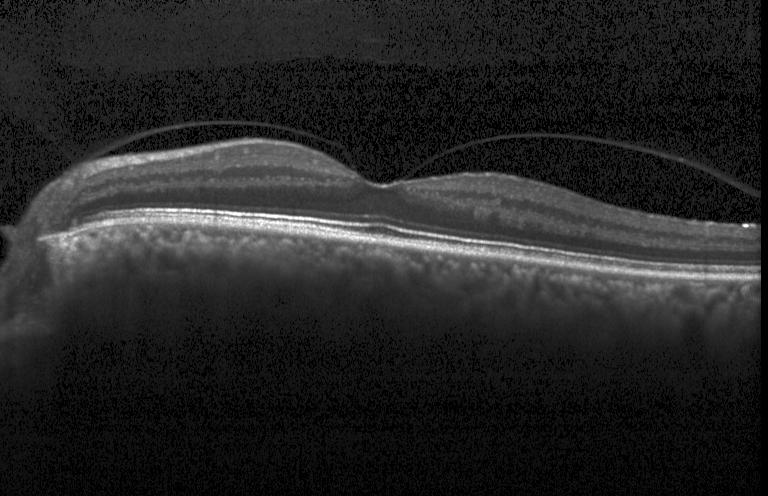 Impression: no CNV, DME, or drusen.